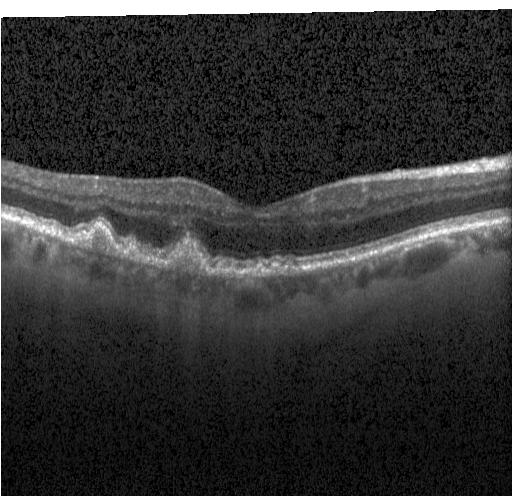
Retinal OCT B-scan, fovea-centered
Macular OCT: multiple drusen.